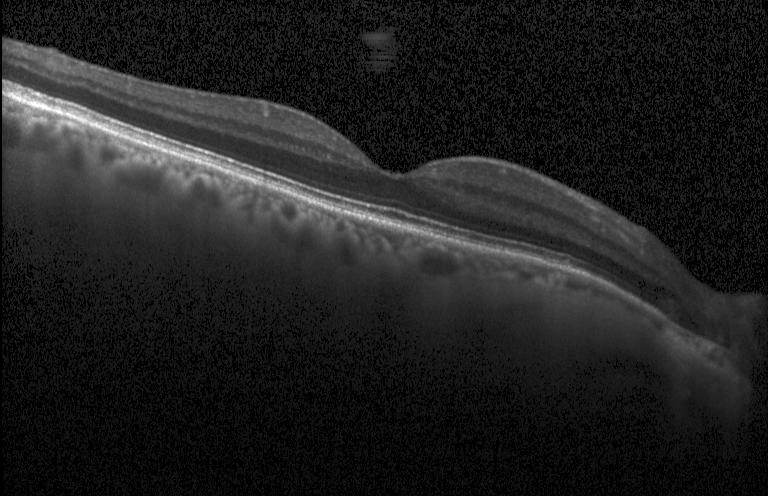
SD-OCT; macular scan; OCT line scan — The scan shows no choroidal neovascularization, no diabetic macular edema, and no drusen.